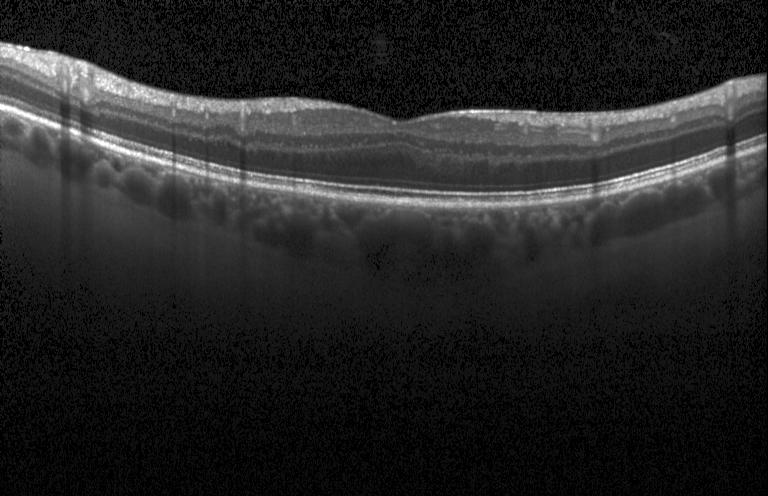 Optical coherence tomography scan; centered on the fovea; spectral-domain OCT.
Impression: neither choroidal neovascularization, diabetic macular edema, nor drusen.